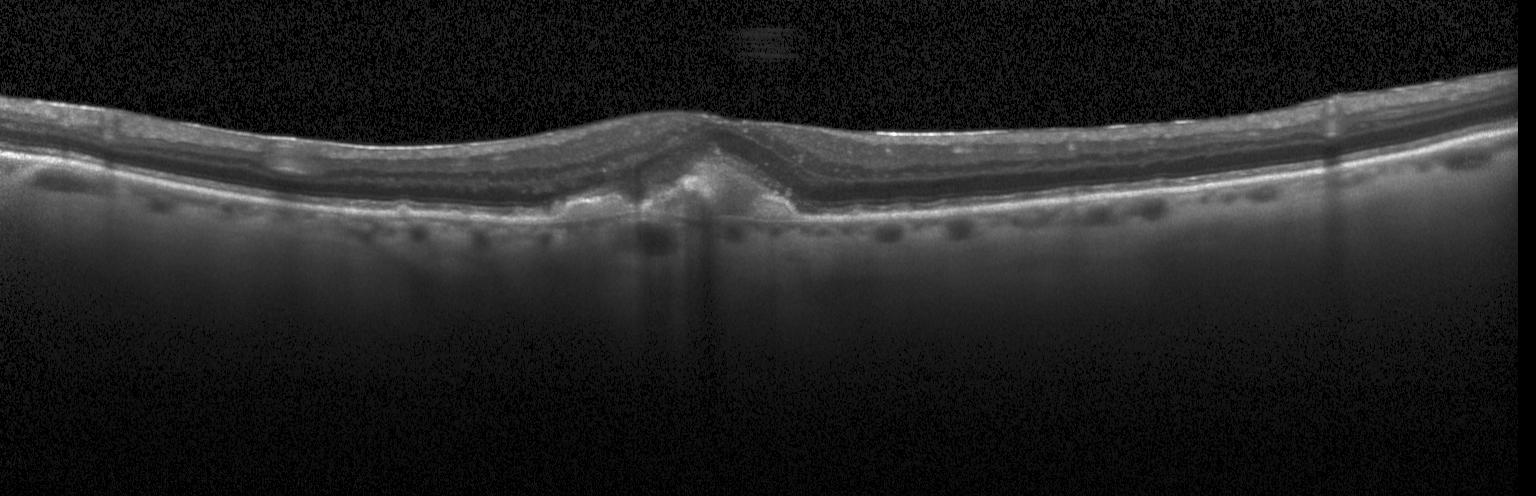
Through the macula · OCT B-scan · spectral-domain optical coherence tomography.
Macular OCT: choroidal neovascularization (CNV).